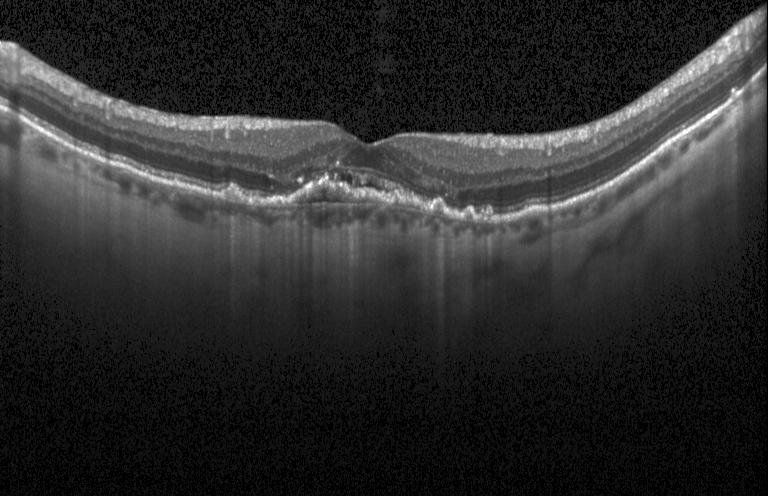
Spectral-domain optical coherence tomography. OCT B-scan.
Diagnosis: CNV.